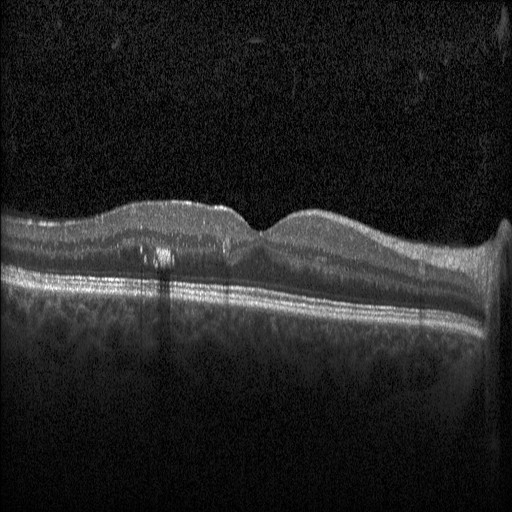 Diabetic macular edema (DME).